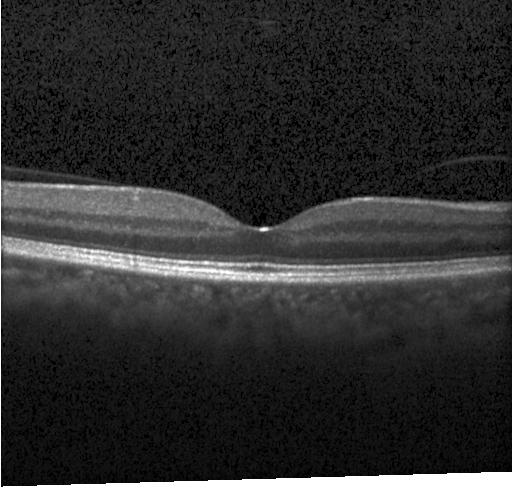
Macular OCT demonstrating no evidence of CNV, DME, or drusen.